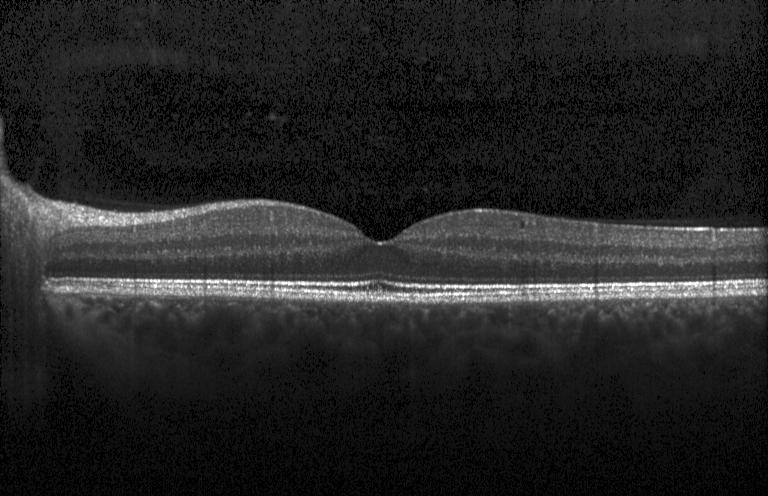 Retinal OCT cross-section · fovea-centered
Finding: neither choroidal neovascularization, diabetic macular edema, nor drusen.